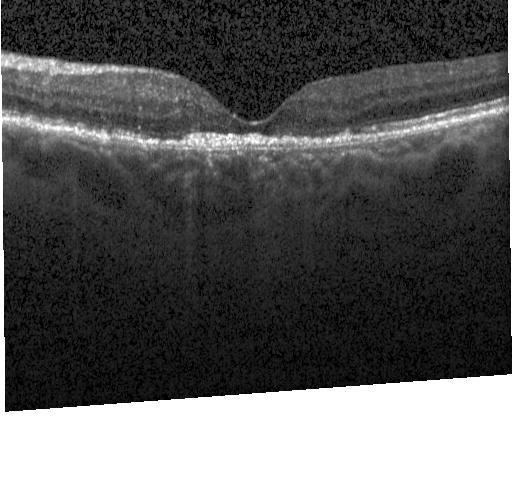 Acquired on a Heidelberg Spectralis, optical coherence tomography B-scan.
Diagnosis: choroidal neovascularization.